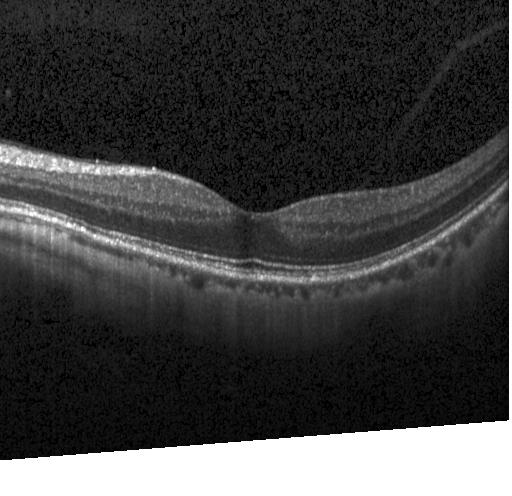 The scan shows no evidence of choroidal neovascularization, diabetic macular edema, or drusen.